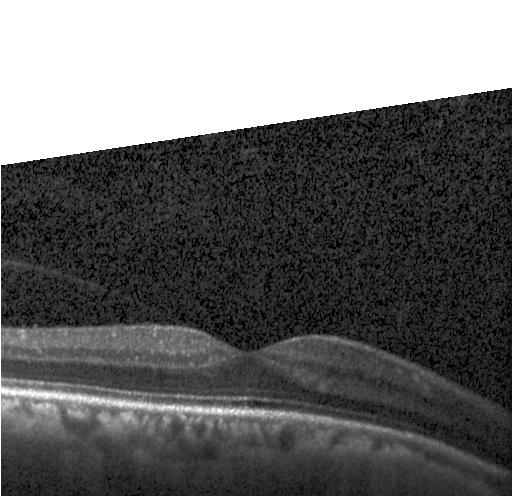 Spectral-domain OCT B-scan: no evidence of choroidal neovascularization, diabetic macular edema, or drusen.